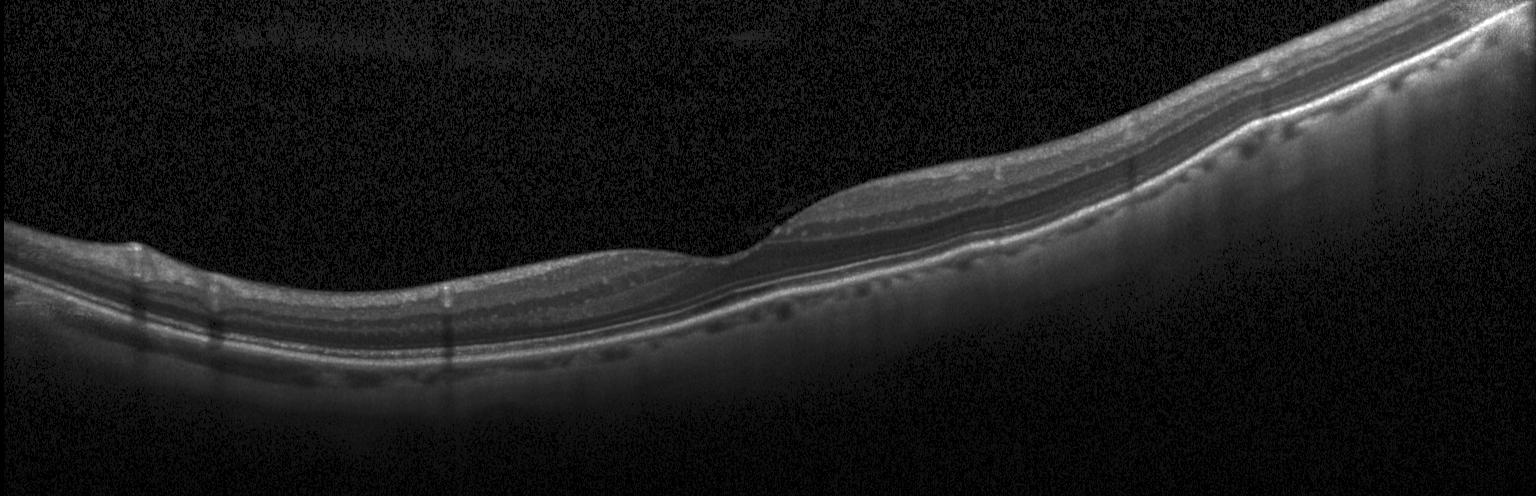
Optical coherence tomography scan.
Assessment: no evidence of CNV, DME, or drusen.